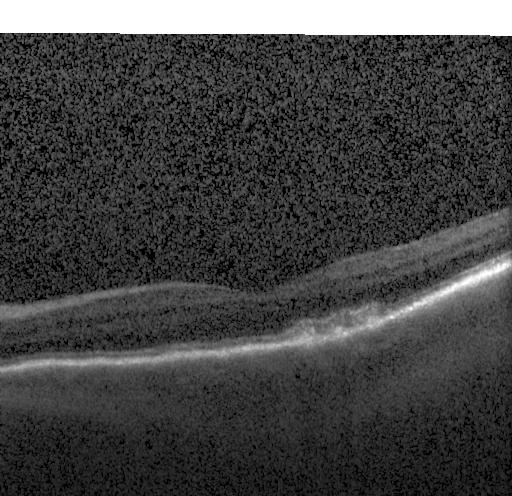 Diagnosis: multiple drusen.